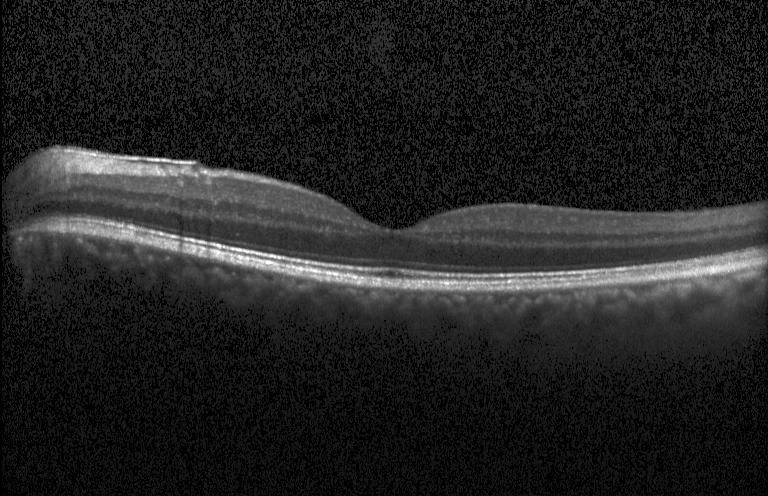
Macular scan. Heidelberg Spectralis OCT system. OCT line scan.
This B-scan demonstrates no choroidal neovascularization, diabetic macular edema, or drusen.